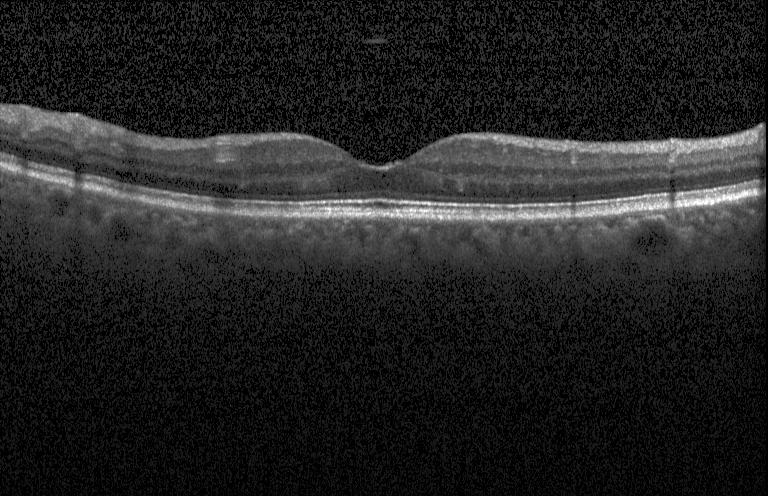
Assessment: neither choroidal neovascularization, diabetic macular edema, nor drusen.